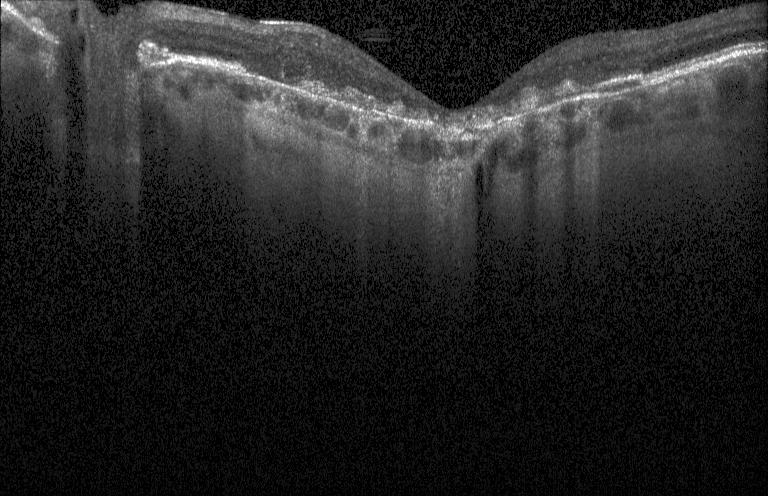
Spectral-domain OCT. Retinal OCT cross-section. Acquired on a Heidelberg Spectralis. This B-scan demonstrates a choroidal neovascular membrane.